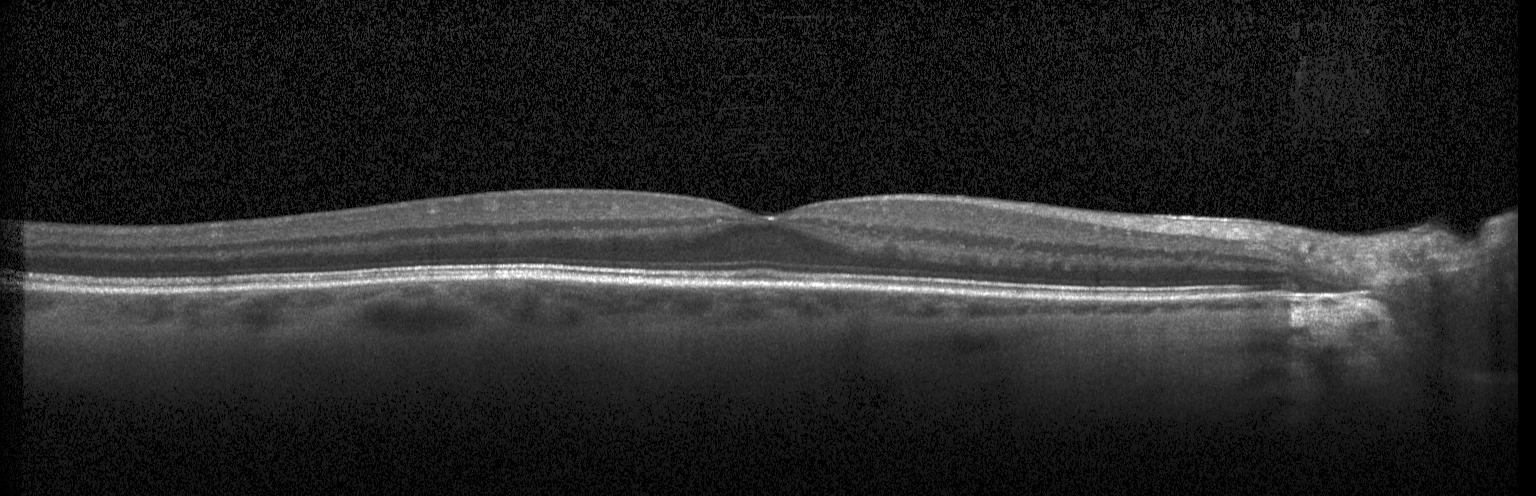 This B-scan demonstrates no choroidal neovascularization, diabetic macular edema, or drusen.